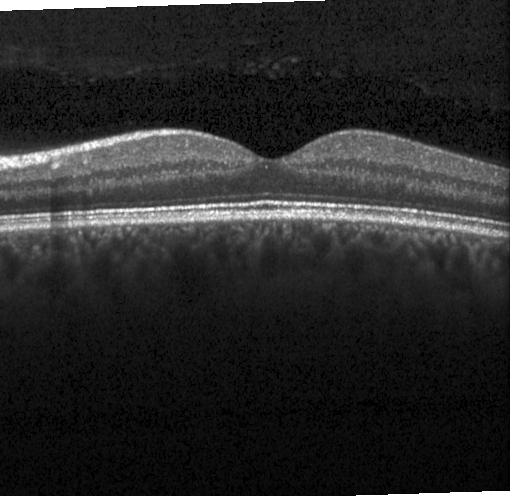
OCT line scan · centered on the fovea · spectral-domain optical coherence tomography · Heidelberg Spectralis.
Assessment: no CNV, DME, or drusen.